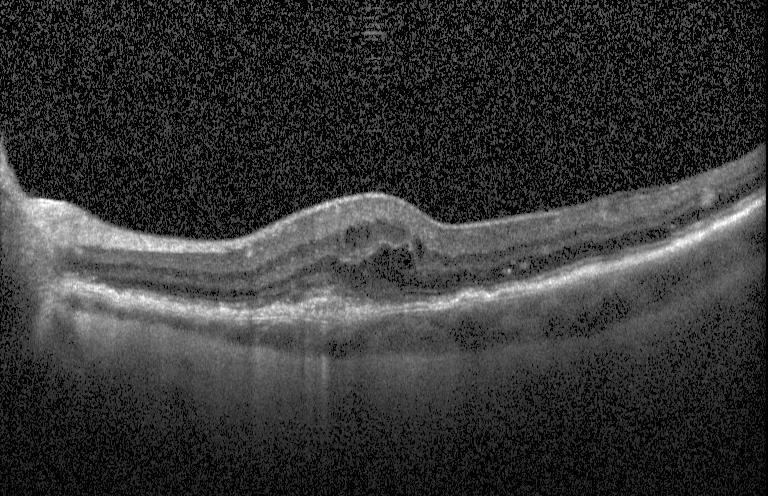
Macular OCT demonstrating CNV.